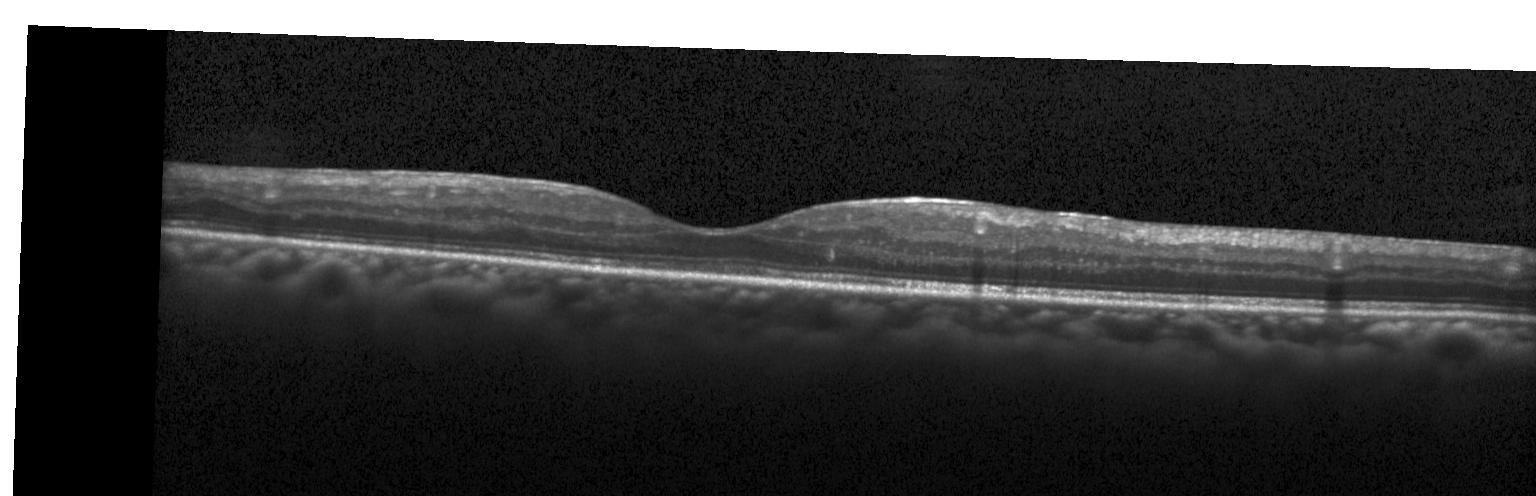
Diagnosis: no evidence of CNV, DME, or drusen.